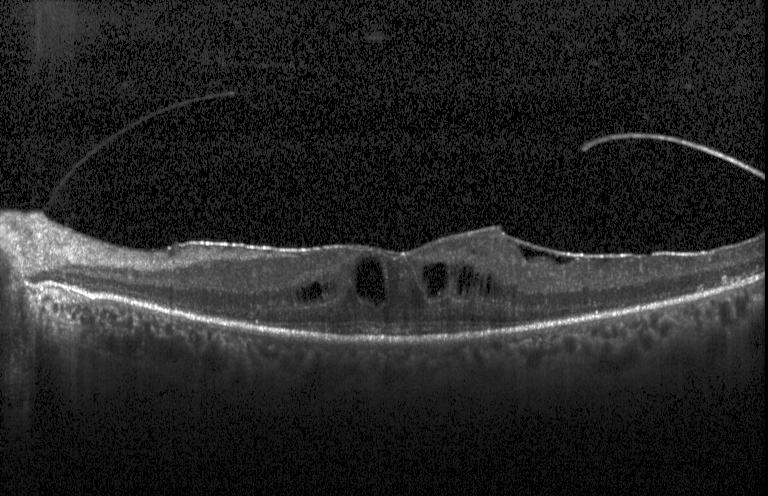

Assessment: diabetic macular edema (DME).